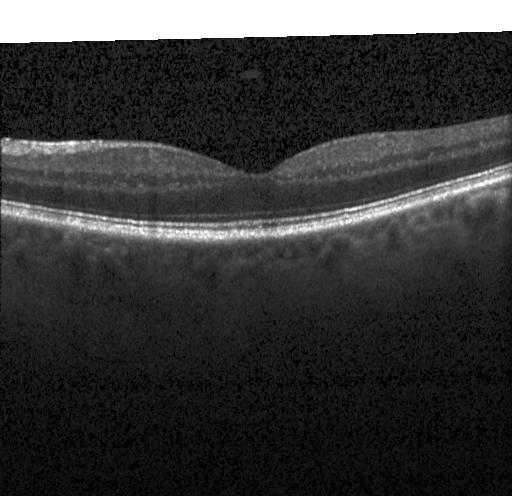 Diagnosis: neither choroidal neovascularization, diabetic macular edema, nor drusen.